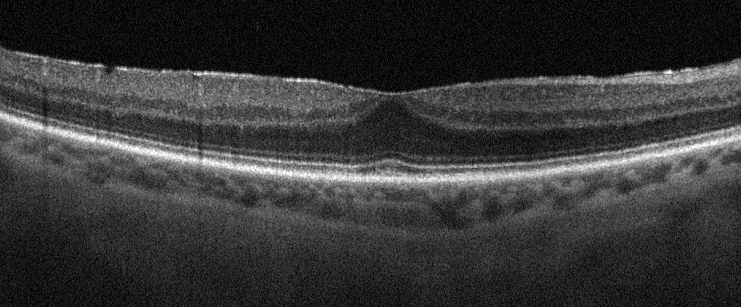 Fovea-centered. Optical coherence tomography scan. Acquired on an Optovue Avanti RTVue XR — Finding: ERM.